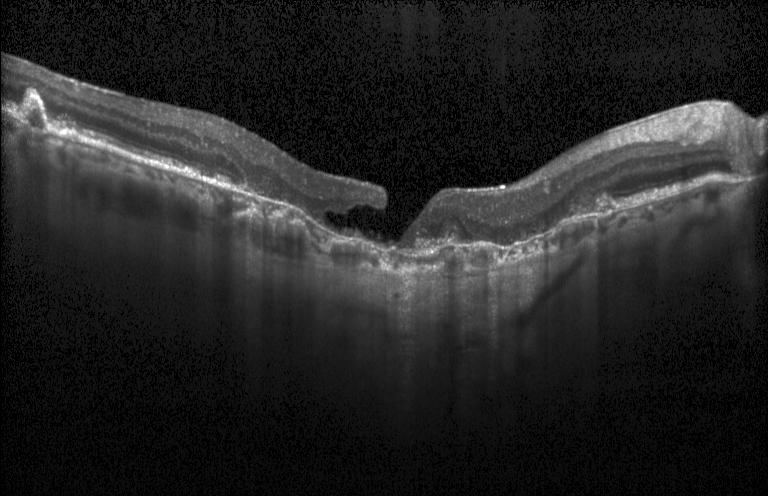

Optical coherence tomography B-scan
The scan shows a choroidal neovascular membrane.